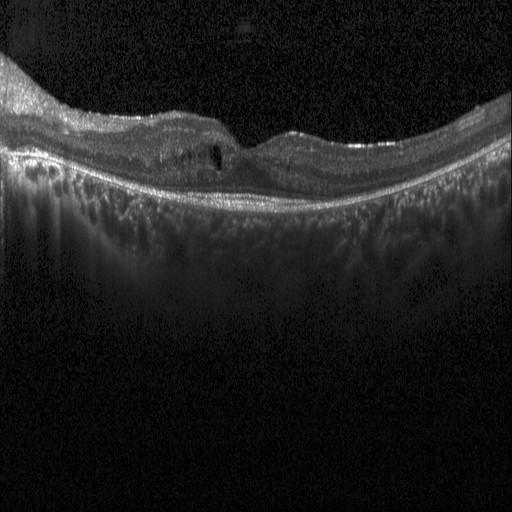 Macular scan · Heidelberg Spectralis OCT system · OCT line scan · spectral-domain optical coherence tomography — DME.